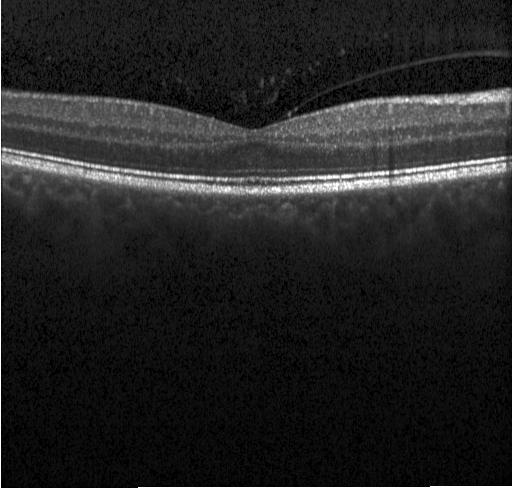

Macular OCT demonstrating no choroidal neovascularization, diabetic macular edema, or drusen.